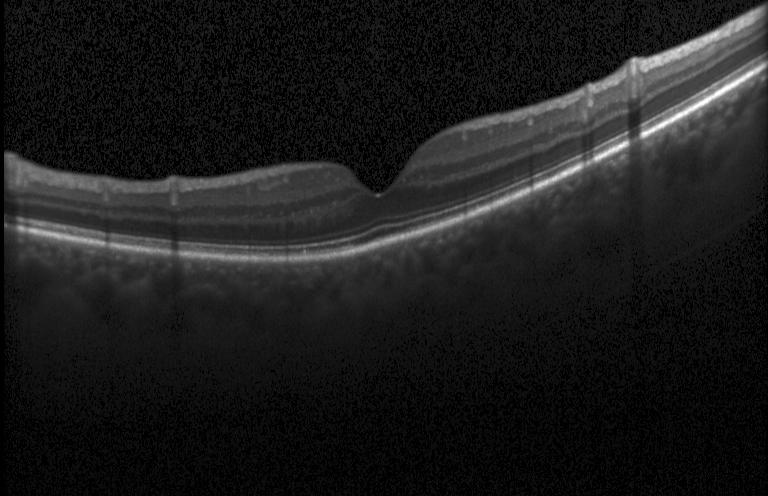

Instrument: Heidelberg Spectralis; optical coherence tomography B-scan; spectral-domain optical coherence tomography; macular scan.
This B-scan demonstrates no choroidal neovascularization, diabetic macular edema, or drusen.